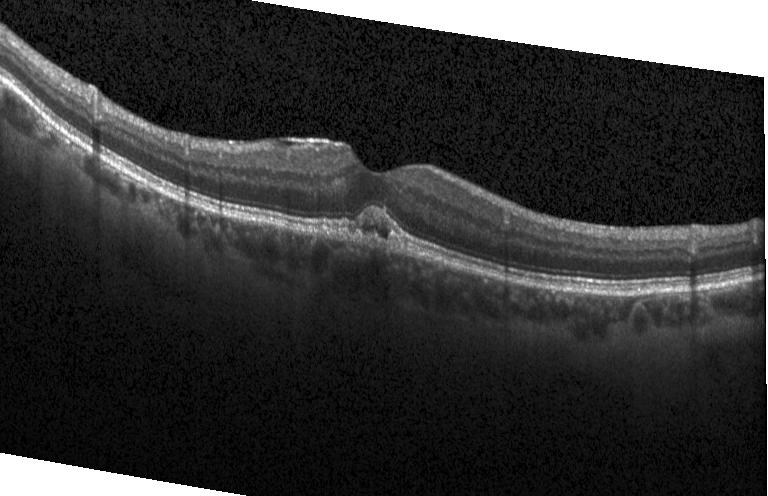
Optical coherence tomography scan. Spectral-domain optical coherence tomography. Heidelberg Spectralis — Finding: choroidal neovascularization.